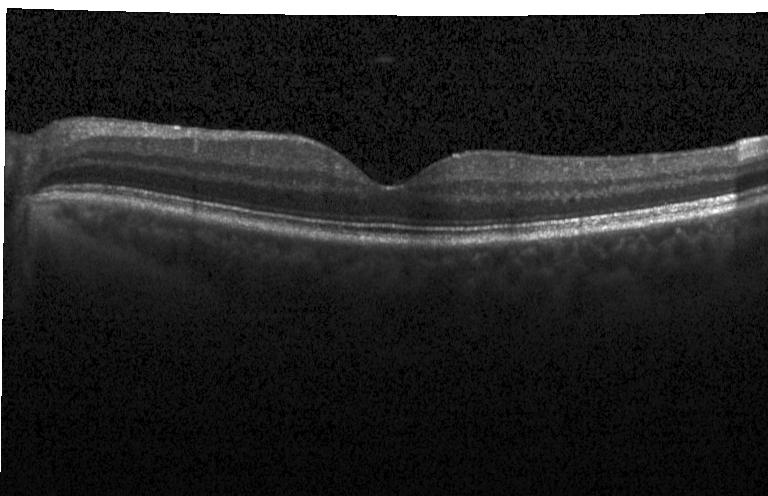 Optical coherence tomography scan.
Finding: no evidence of choroidal neovascularization, diabetic macular edema, or drusen.